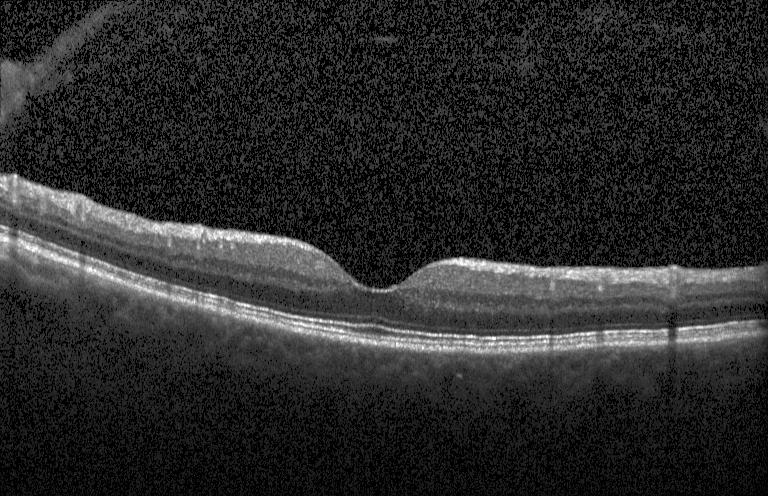

Optical coherence tomography B-scan
Diagnosis: no choroidal neovascularization, no diabetic macular edema, and no drusen.